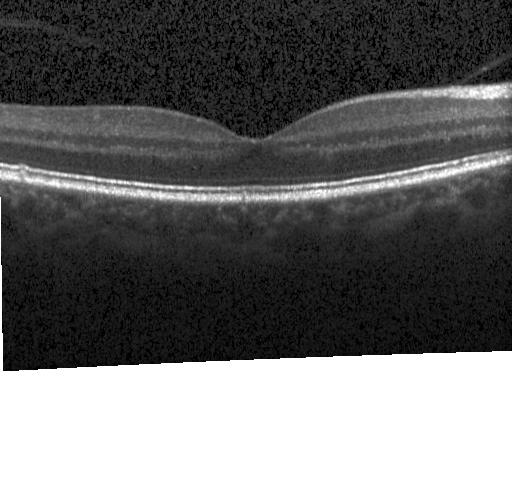

Optical coherence tomography scan. Drusen.